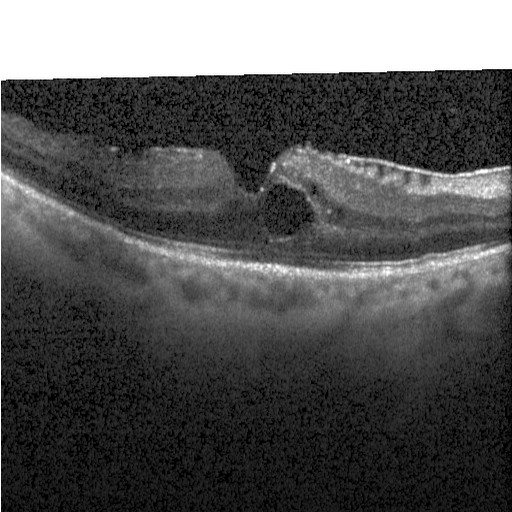
OCT line scan, through the macula, acquired on a Heidelberg Spectralis, spectral-domain OCT
Macular OCT: diabetic macular edema (DME).